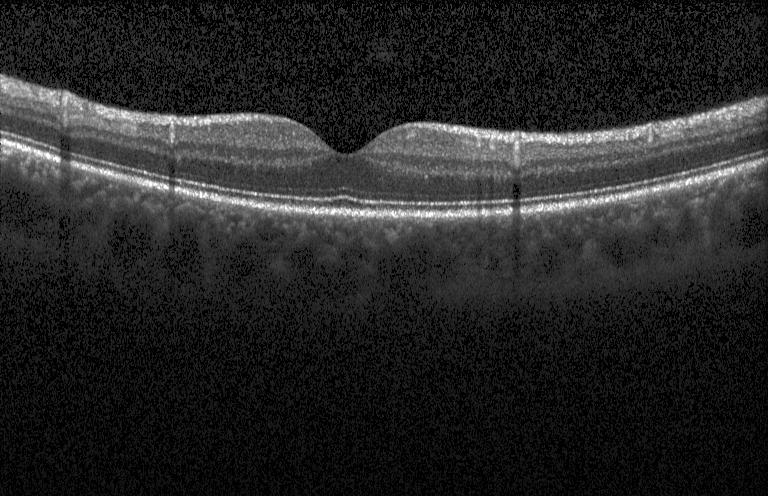 Dx: no choroidal neovascularization, diabetic macular edema, or drusen.